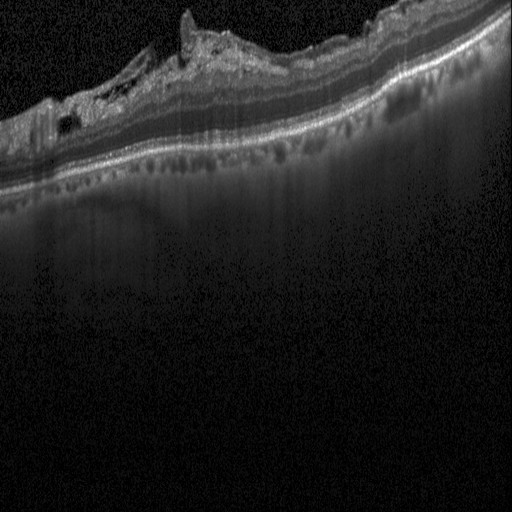
This B-scan demonstrates diabetic macular edema (DME).